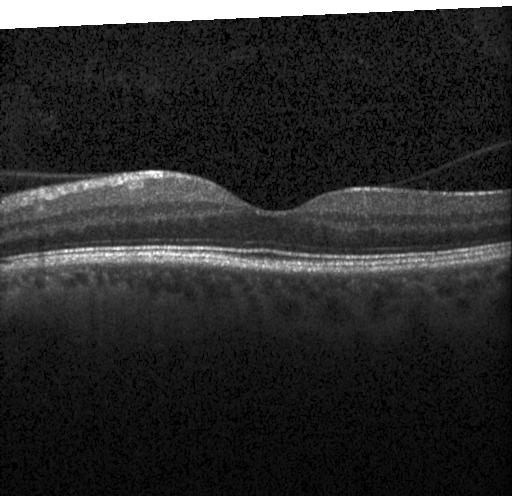 Macular scan, spectral-domain OCT, Heidelberg Spectralis OCT system, optical coherence tomography B-scan — Finding: neither CNV, DME, nor drusen.